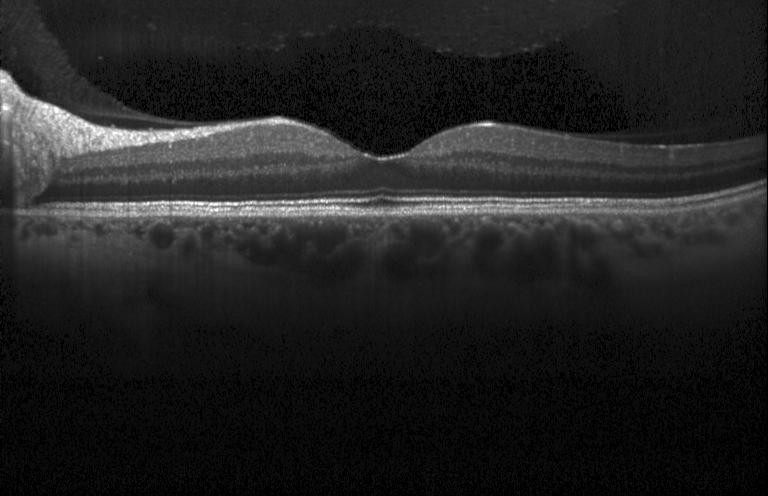

Spectral-domain OCT B-scan: no evidence of CNV, DME, or drusen.